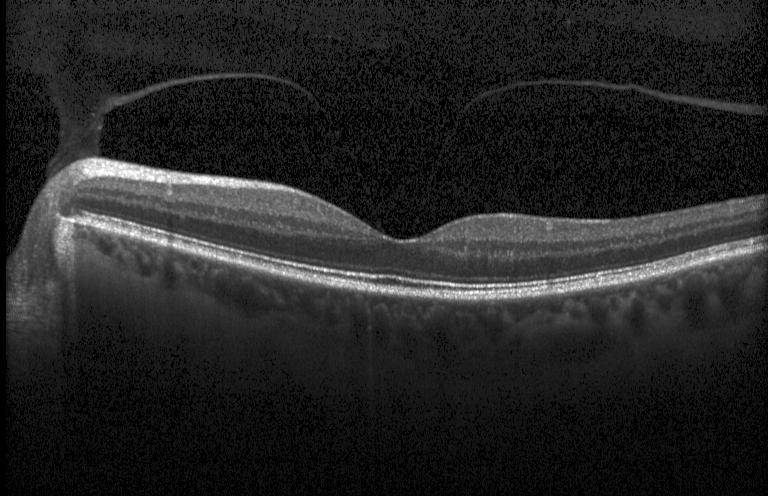 OCT line scan; macular scan. Impression: no choroidal neovascularization, diabetic macular edema, or drusen.